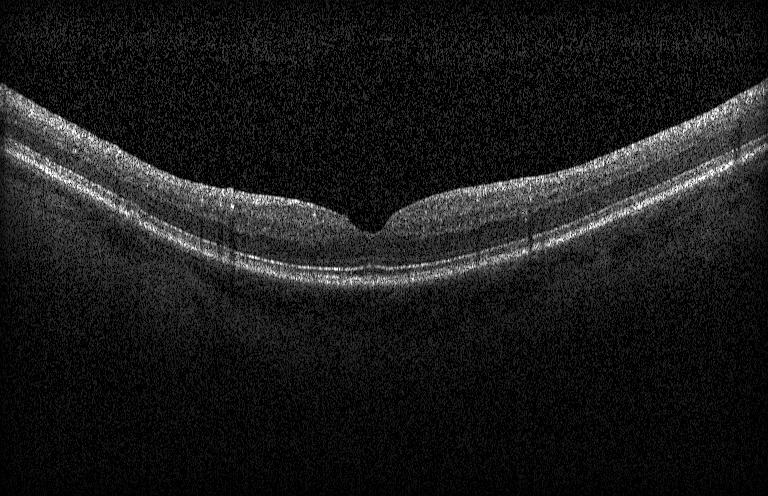 OCT line scan. Spectral-domain OCT. Diagnosis: no choroidal neovascularization, no diabetic macular edema, and no drusen.